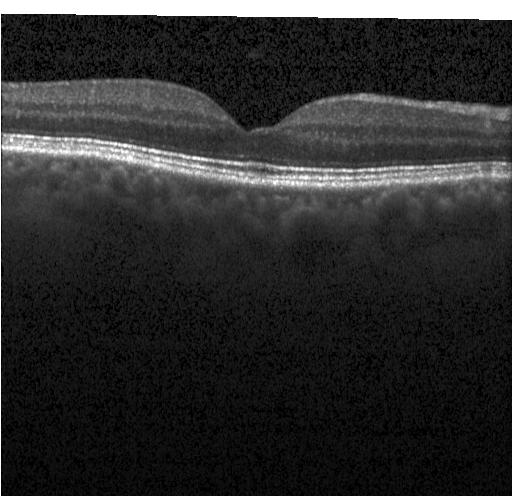

OCT B-scan showing neither choroidal neovascularization, diabetic macular edema, nor drusen.